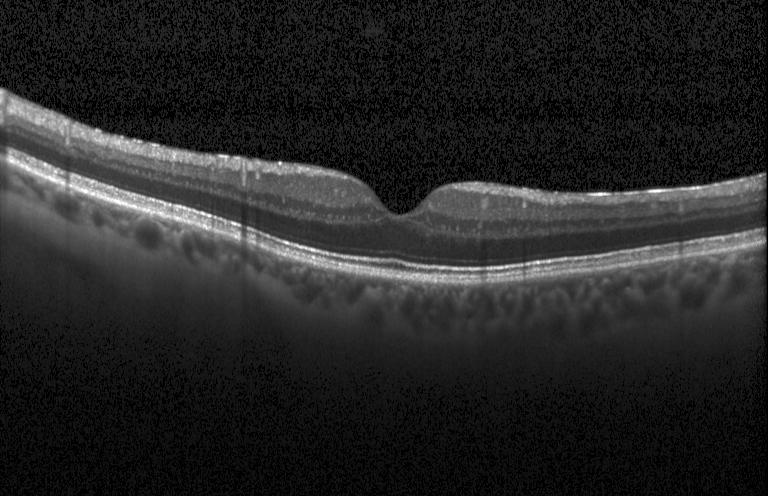

The scan shows no choroidal neovascularization, no diabetic macular edema, and no drusen.